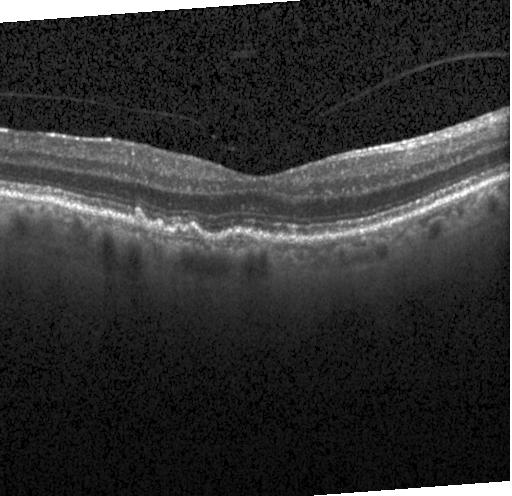 Finding: drusen.